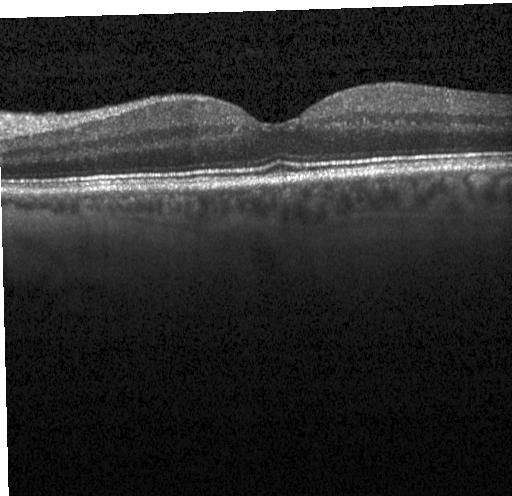 Impression: no choroidal neovascularization, no diabetic macular edema, and no drusen.